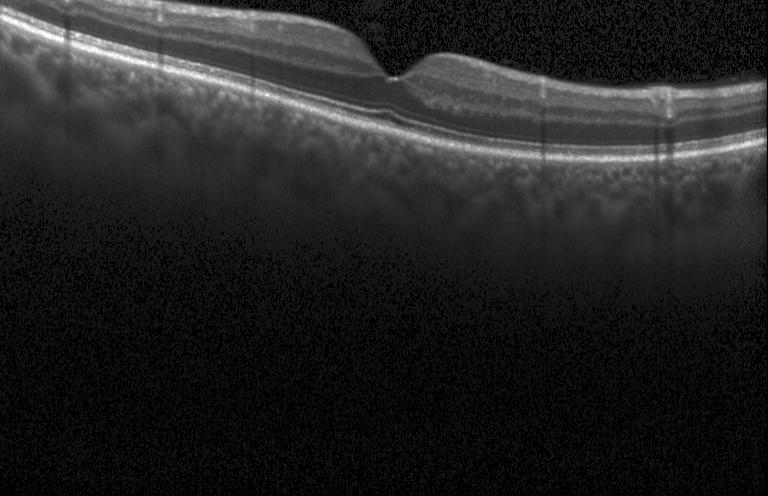

Retinal OCT cross-section, spectral-domain OCT
The scan shows no CNV, DME, or drusen.